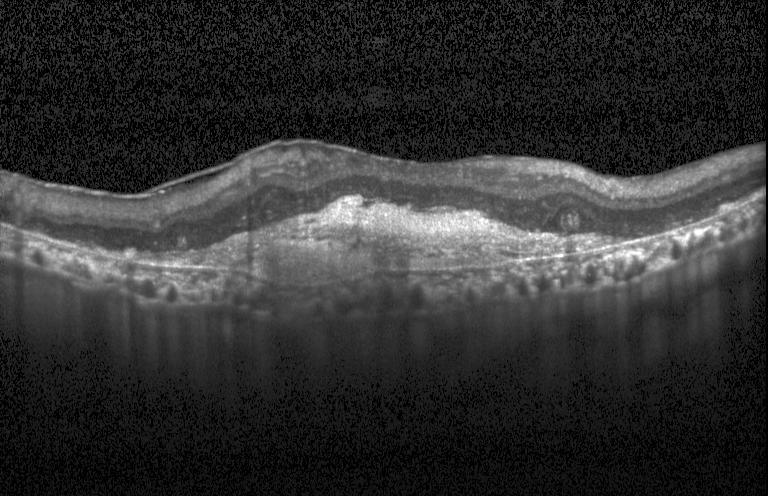 Retinal OCT B-scan. Dx: a choroidal neovascular membrane.